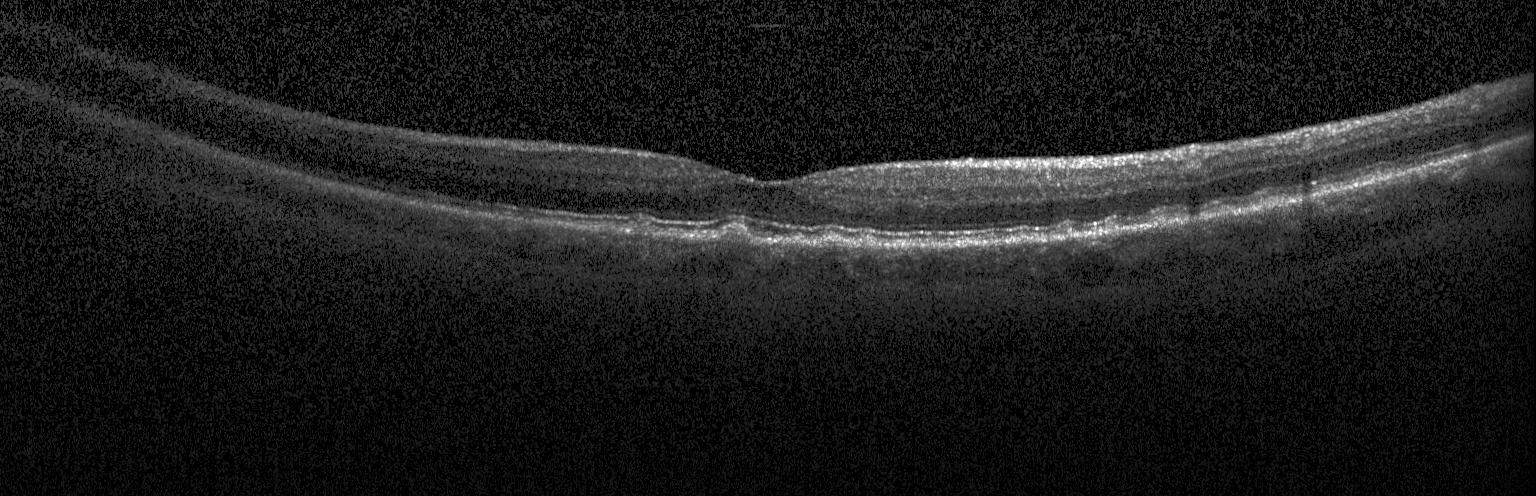

Heidelberg Spectralis, retinal OCT B-scan, through the macula — Impression: drusen.